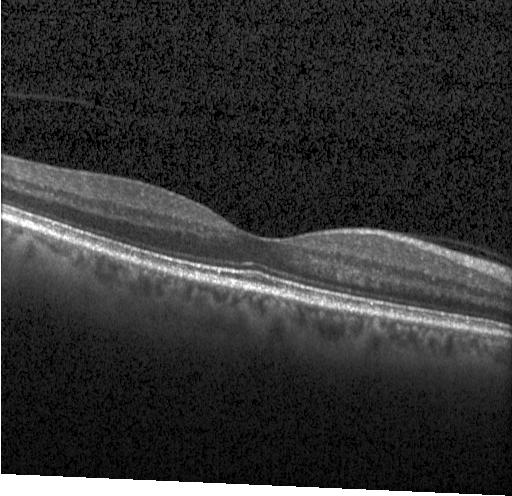 Macular OCT: no choroidal neovascularization, no diabetic macular edema, and no drusen.